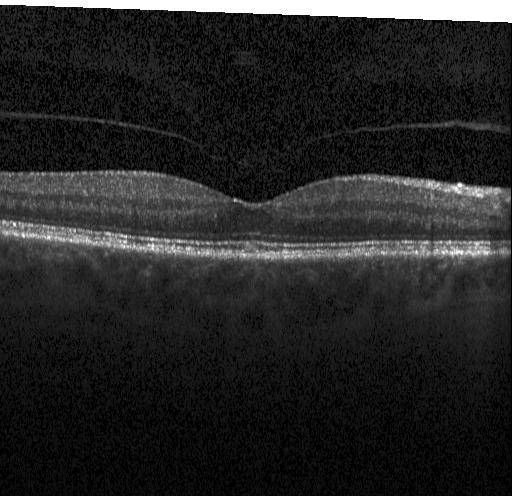 This B-scan demonstrates no choroidal neovascularization, no diabetic macular edema, and no drusen.